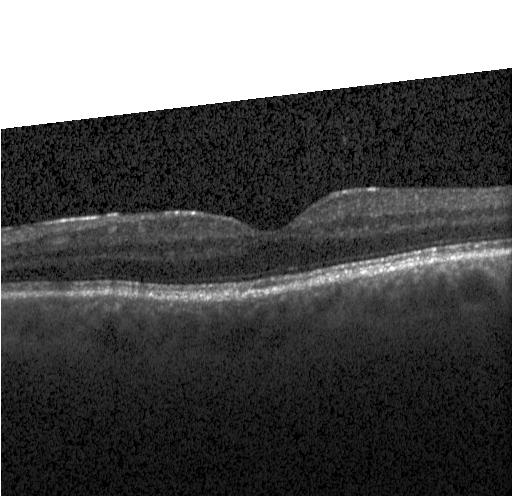

OCT B-scan showing neither choroidal neovascularization, diabetic macular edema, nor drusen.